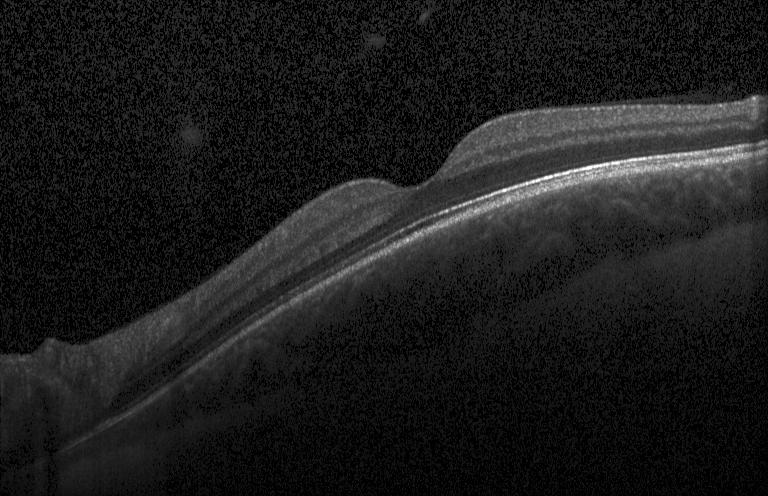
SD-OCT · OCT B-scan
This B-scan demonstrates no evidence of choroidal neovascularization, diabetic macular edema, or drusen.